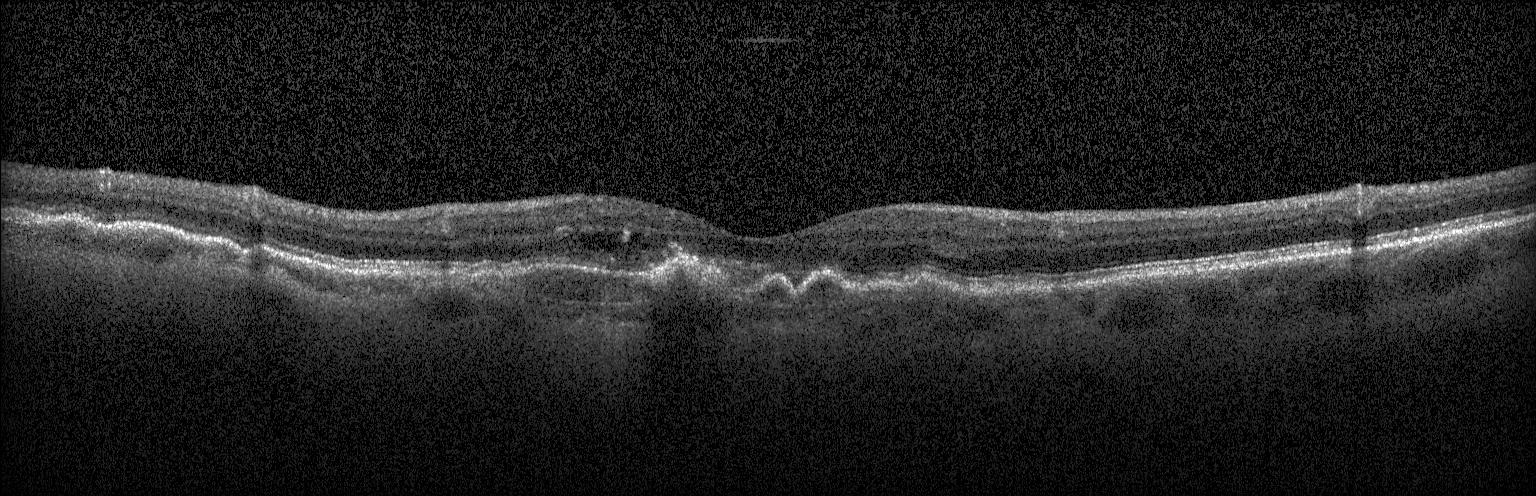 Acquired on a Heidelberg Spectralis, optical coherence tomography scan. Impression: CNV.